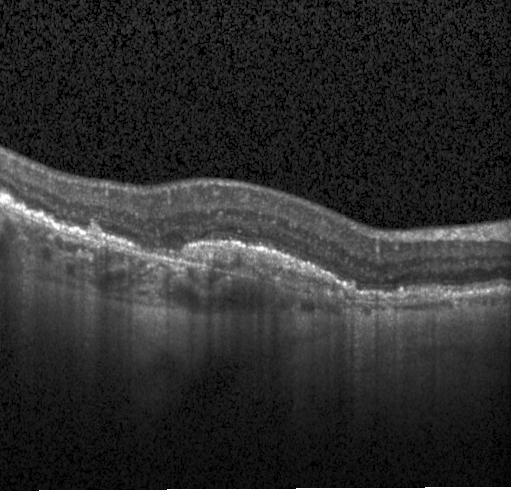 Heidelberg Spectralis OCT system, through the macula, optical coherence tomography B-scan, SD-OCT.
Diagnosis: CNV.